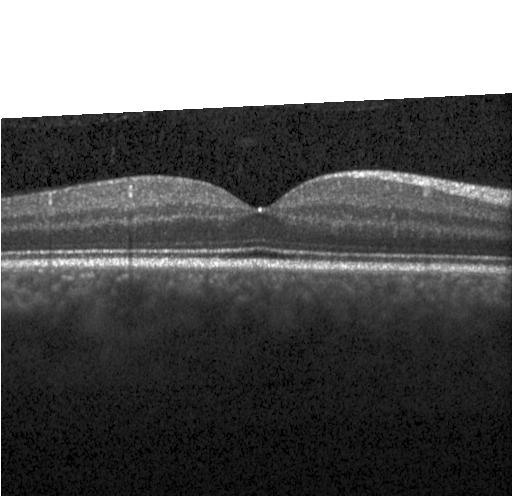

The scan shows no choroidal neovascularization, diabetic macular edema, or drusen.